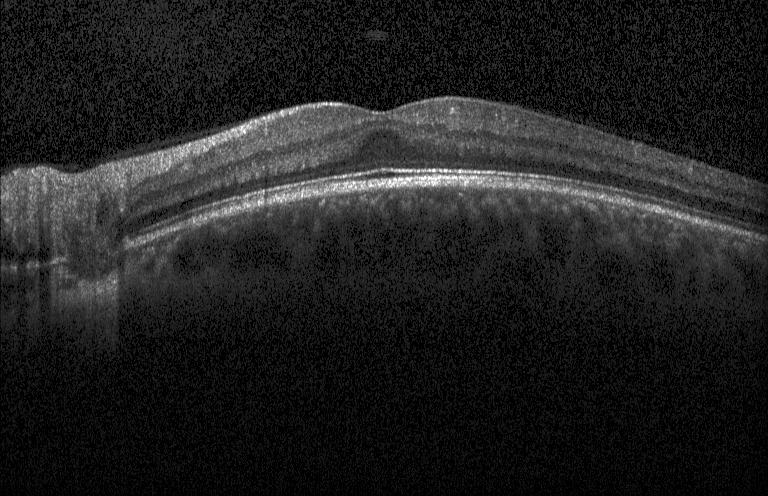 OCT finding: no choroidal neovascularization, diabetic macular edema, or drusen.